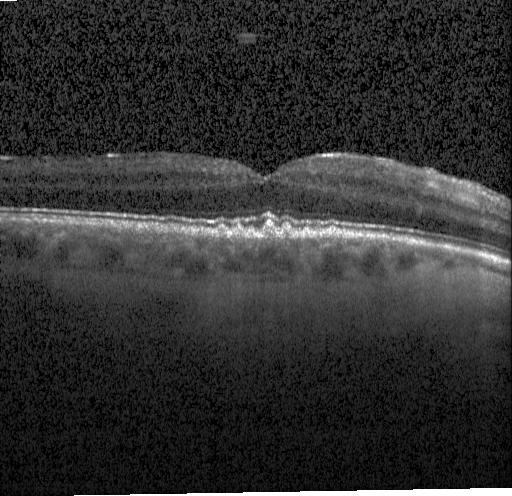

OCT scan showing drusen.